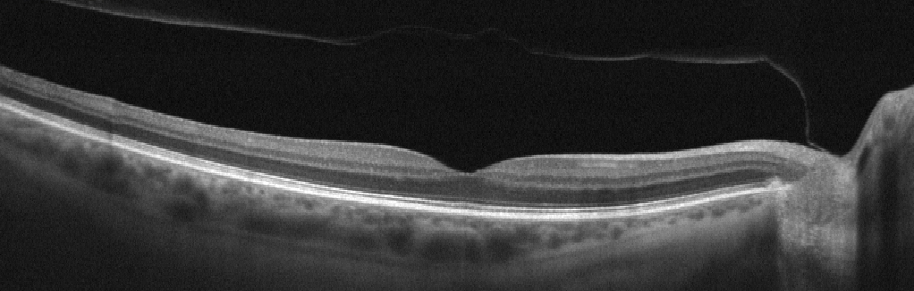

Oculus dexter, optical coherence tomography scan. Finding: absence of AMD, DME, ERM, RAO, RVO, and vitreomacular interface disease.